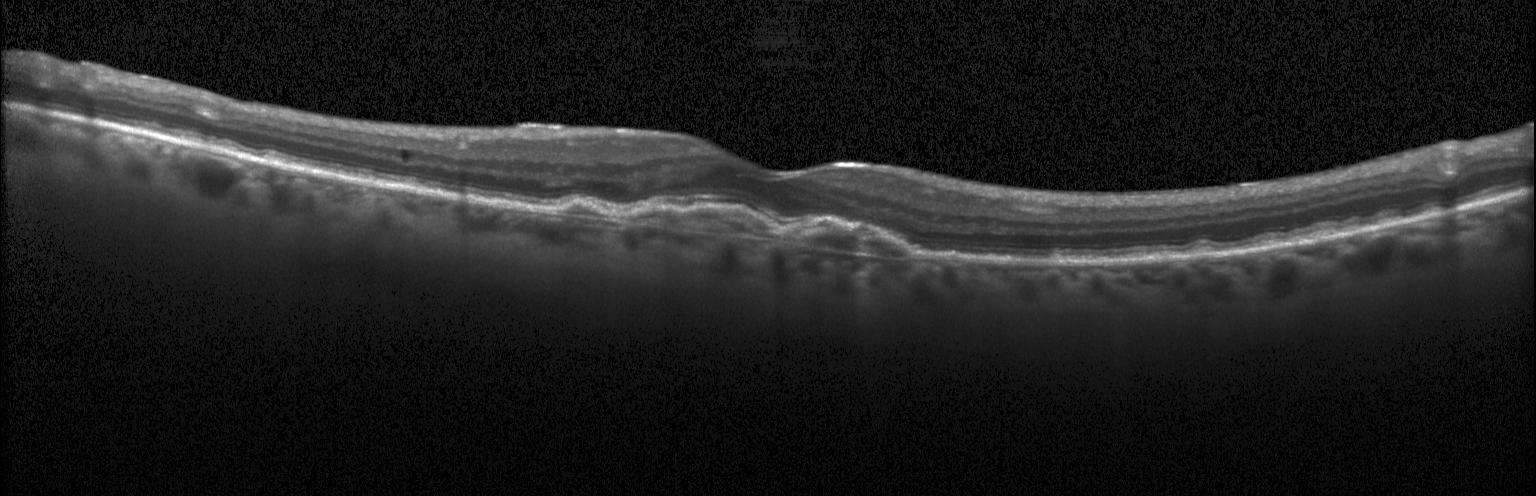 Impression: choroidal neovascularization (CNV).